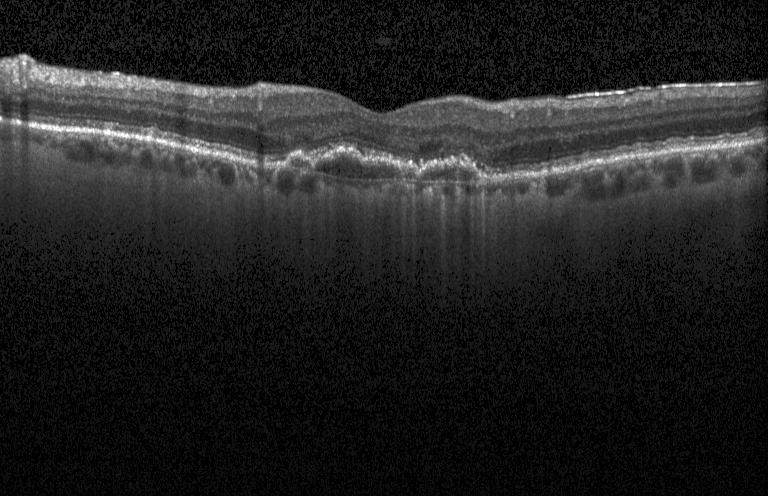
Horizontal scan through the fovea. Optical coherence tomography scan.
Dx: CNV.